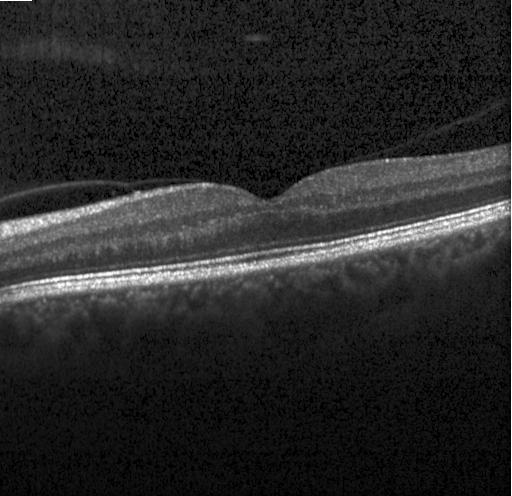

Fovea-centered, spectral-domain optical coherence tomography, optical coherence tomography B-scan, instrument: Heidelberg Spectralis.
Diagnosis: no evidence of CNV, DME, or drusen.